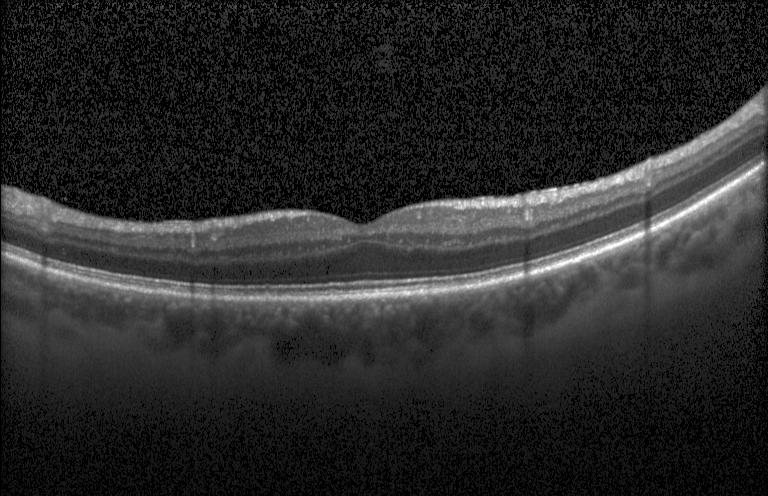
Retinal OCT cross-section
Finding: no evidence of choroidal neovascularization, diabetic macular edema, or drusen.